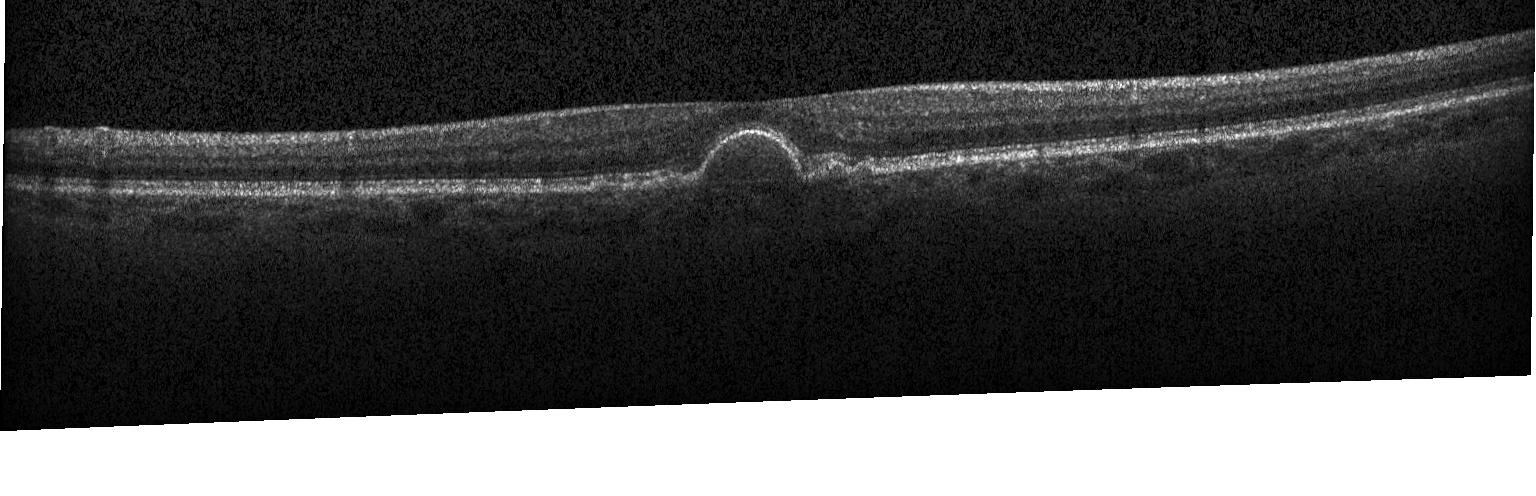

Optical coherence tomography B-scan
Finding: a choroidal neovascular membrane.